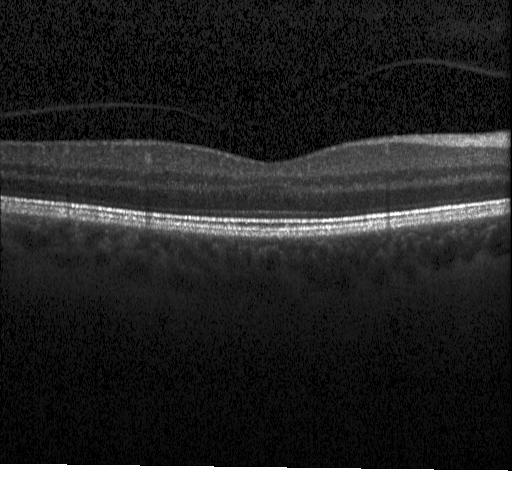 OCT B-scan; spectral-domain optical coherence tomography; horizontal scan through the fovea; instrument: Heidelberg Spectralis. Finding: neither CNV, DME, nor drusen.